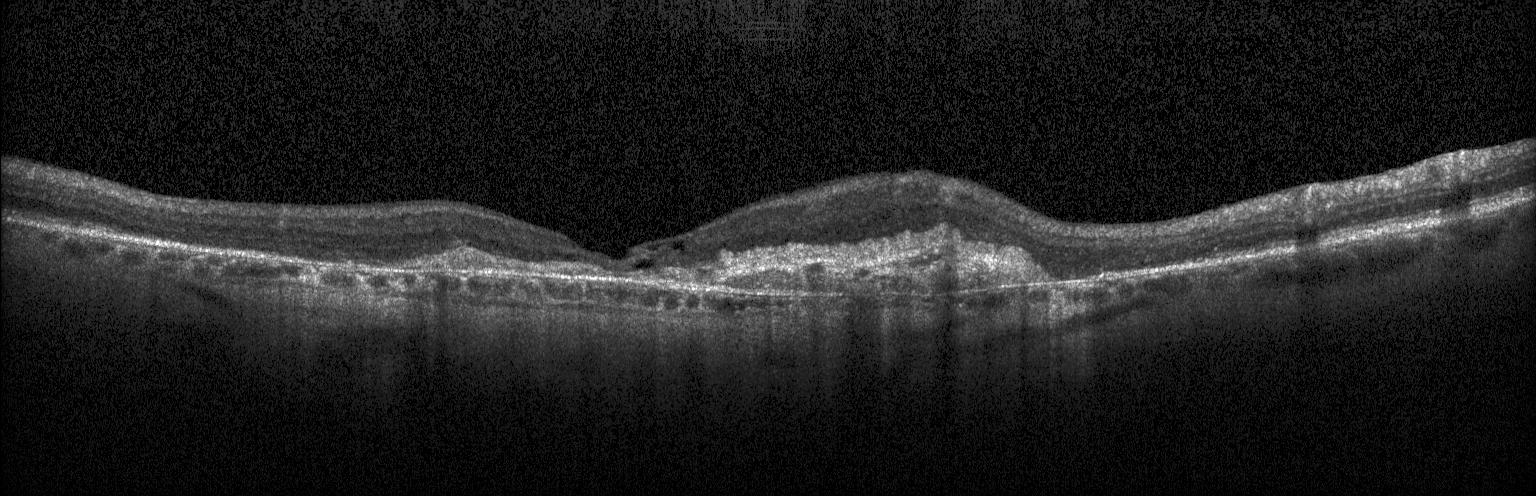

Optical coherence tomography B-scan. This B-scan demonstrates choroidal neovascularization (CNV).